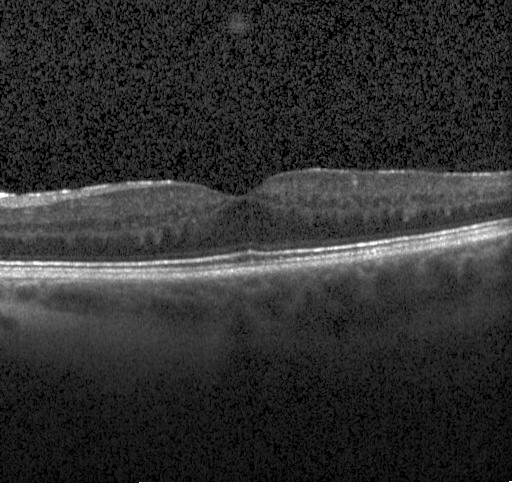

Retinal OCT cross-section. Horizontal scan through the fovea — This B-scan demonstrates no choroidal neovascularization, no diabetic macular edema, and no drusen.